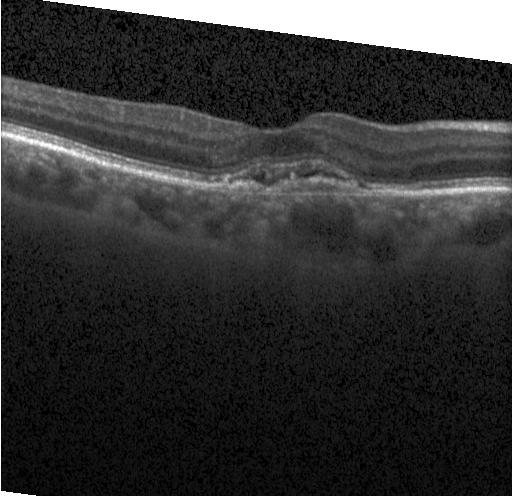

Spectral-domain OCT; Heidelberg Spectralis OCT system; retinal OCT cross-section; through the macula. Macular OCT: choroidal neovascularization.